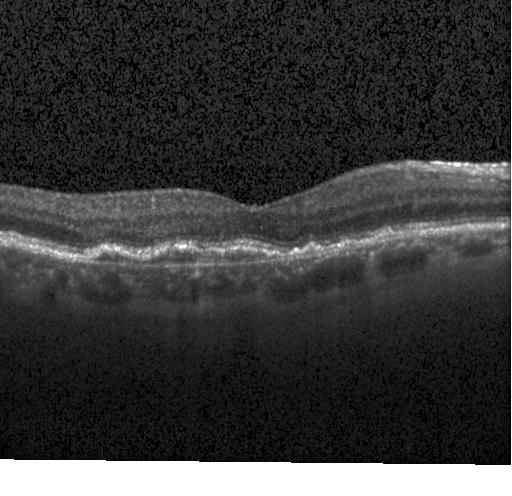

Optical coherence tomography scan. Heidelberg Spectralis OCT system. Horizontal scan through the fovea. Diagnosis: a choroidal neovascular membrane.